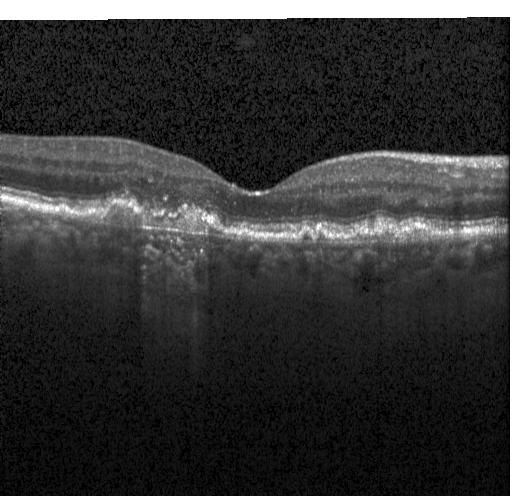
Retinal OCT cross-section. A choroidal neovascular membrane.